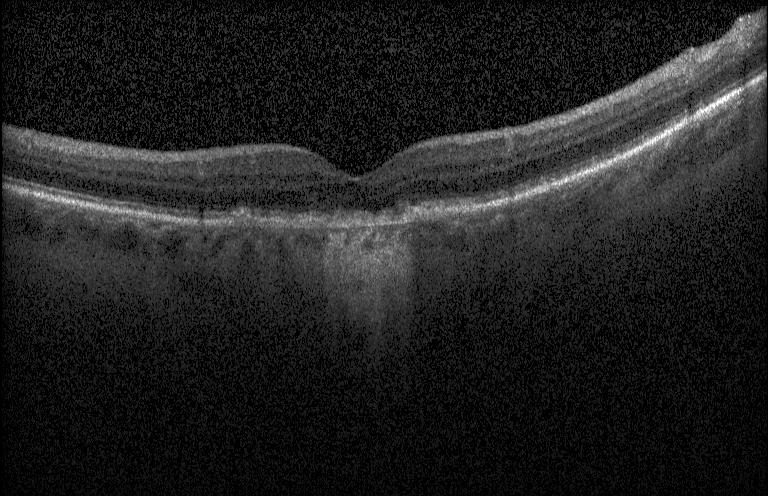
Dx: a choroidal neovascular membrane.